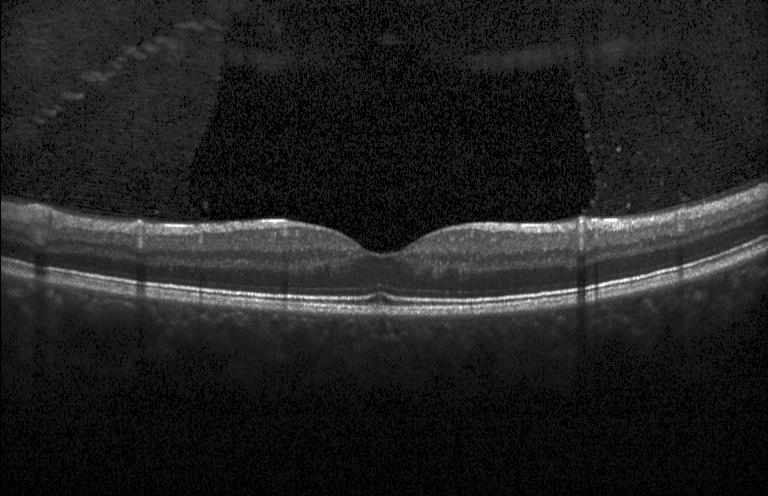

Optical coherence tomography scan; acquired on a Heidelberg Spectralis
Diagnosis: no evidence of CNV, DME, or drusen.